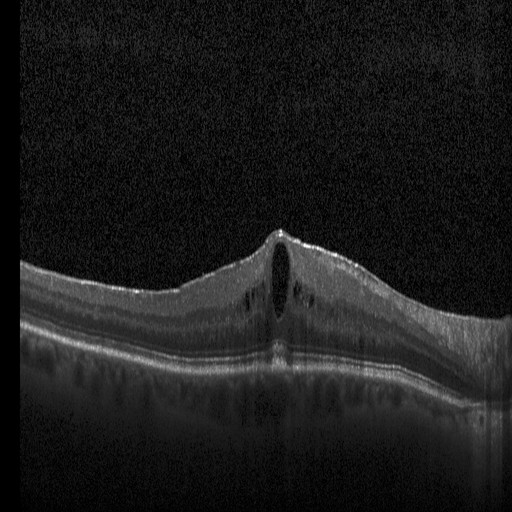
Retinal OCT cross-section.
Dx: diabetic macular edema (DME).